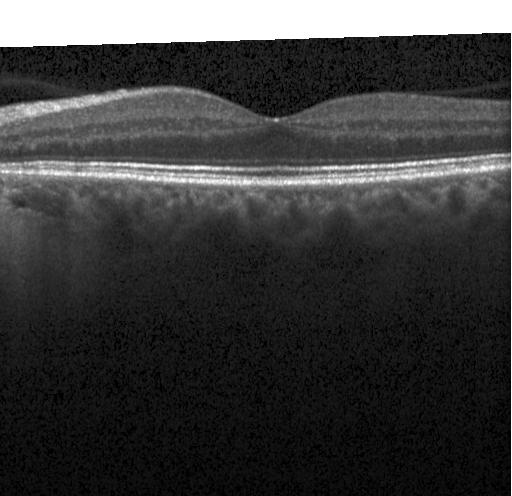
Macular OCT demonstrating neither choroidal neovascularization, diabetic macular edema, nor drusen.